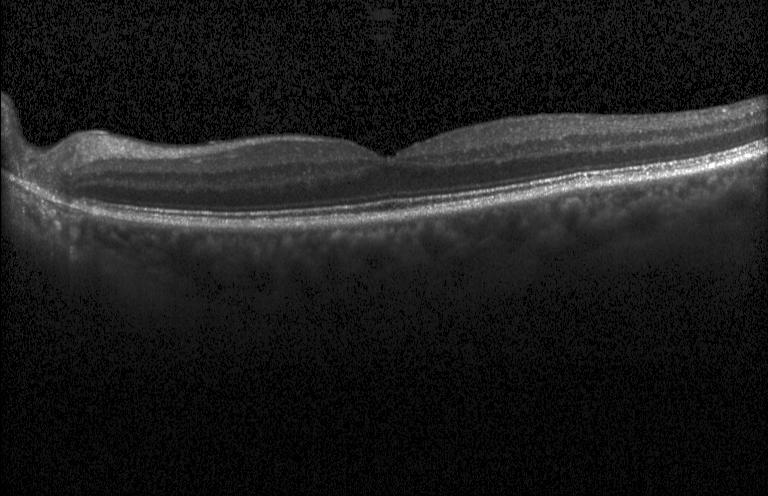
Impression: neither choroidal neovascularization, diabetic macular edema, nor drusen.